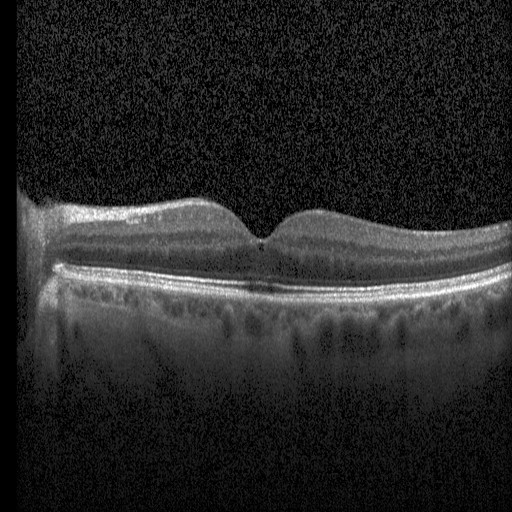

Retinal OCT B-scan. Acquired on a Heidelberg Spectralis. Fovea-centered. SD-OCT.
Diagnosis: DME.